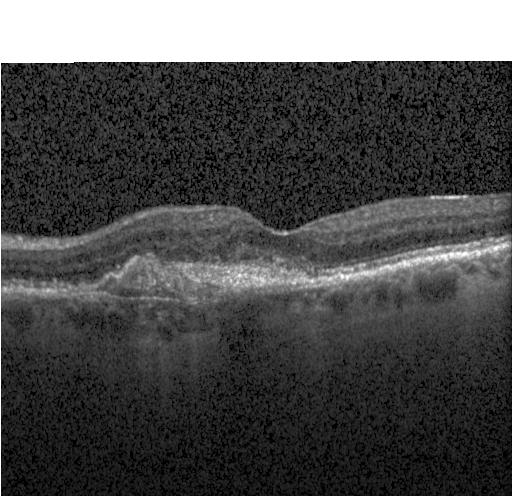

Optical coherence tomography scan — Finding: choroidal neovascularization.